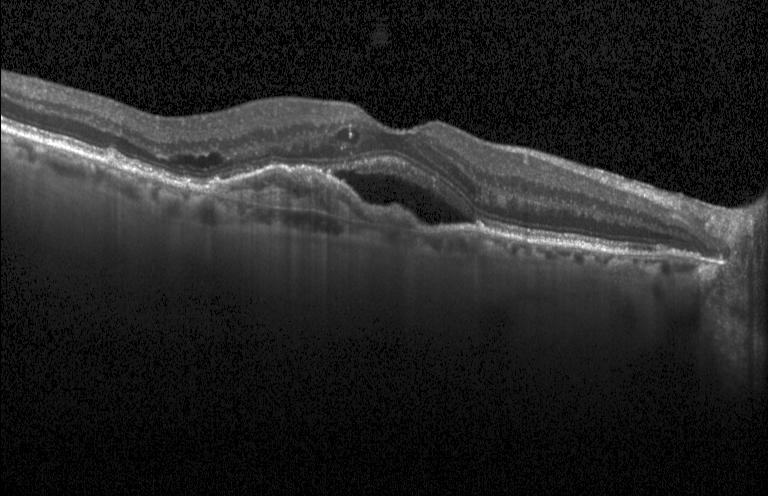

Horizontal scan through the fovea, retinal OCT B-scan, Heidelberg Spectralis. Finding: CNV.